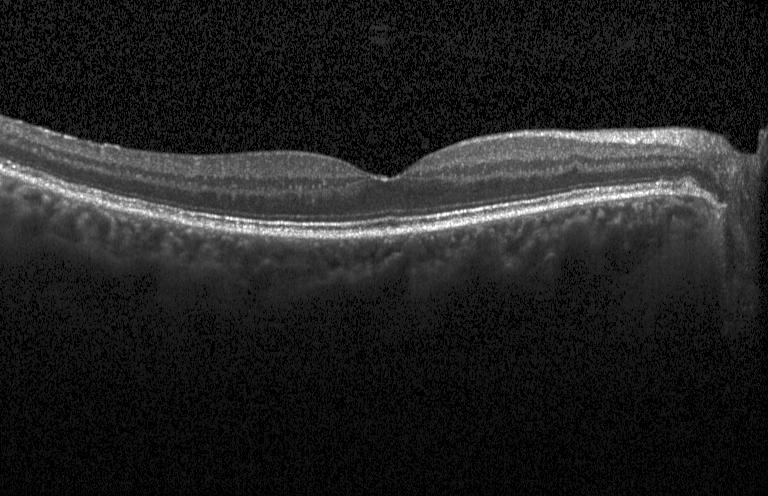

Through the macula · optical coherence tomography scan
Finding: no choroidal neovascularization, no diabetic macular edema, and no drusen.